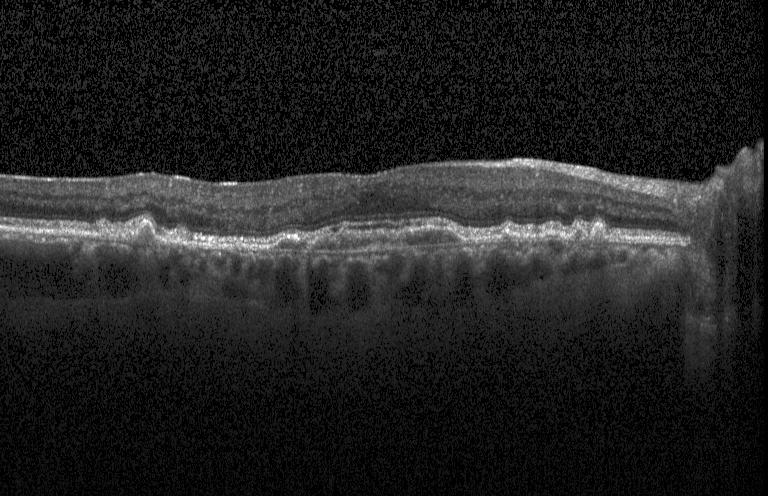
Macular OCT demonstrating choroidal neovascularization (CNV).